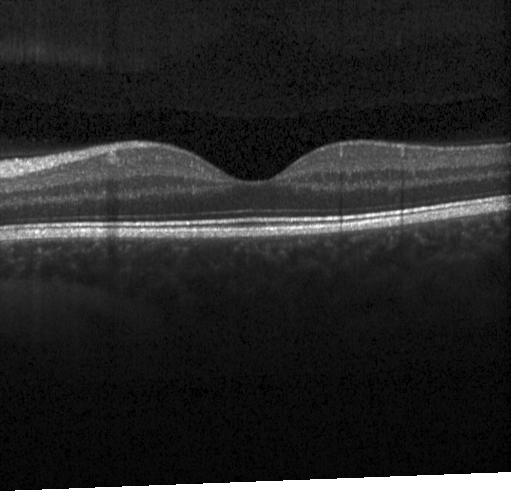

OCT line scan · spectral-domain optical coherence tomography. OCT finding: no choroidal neovascularization, diabetic macular edema, or drusen.